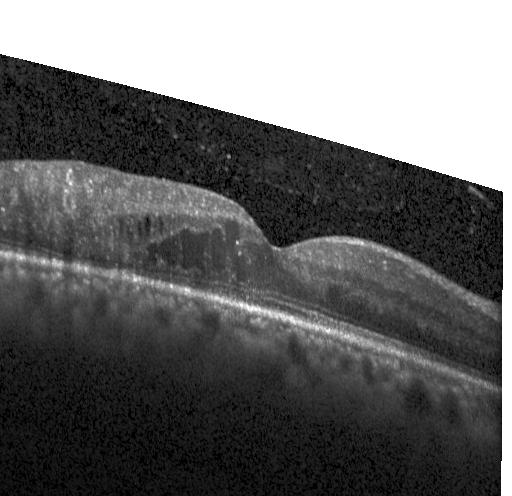 Spectral-domain OCT. Optical coherence tomography scan. Macular scan — Dx: DME.